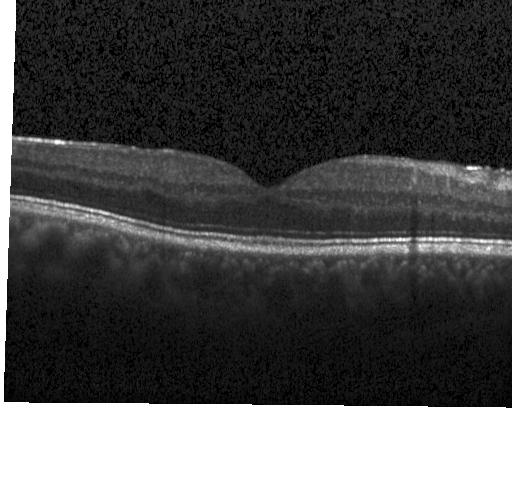

Macular OCT: no choroidal neovascularization, diabetic macular edema, or drusen.